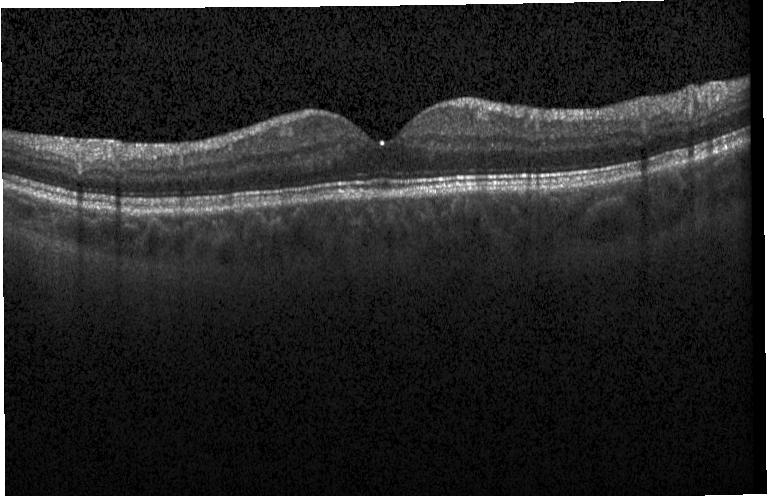

Assessment: neither choroidal neovascularization, diabetic macular edema, nor drusen.